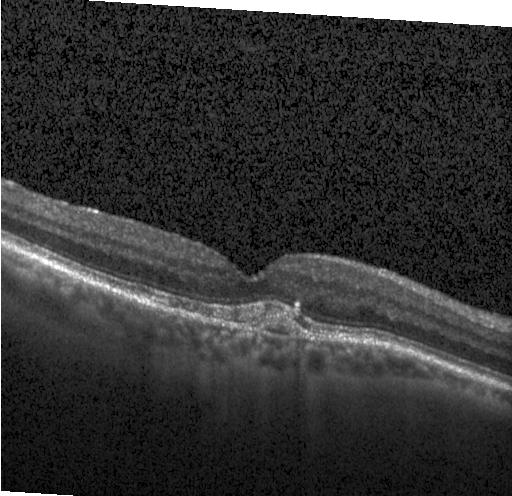 Finding: choroidal neovascularization (CNV).